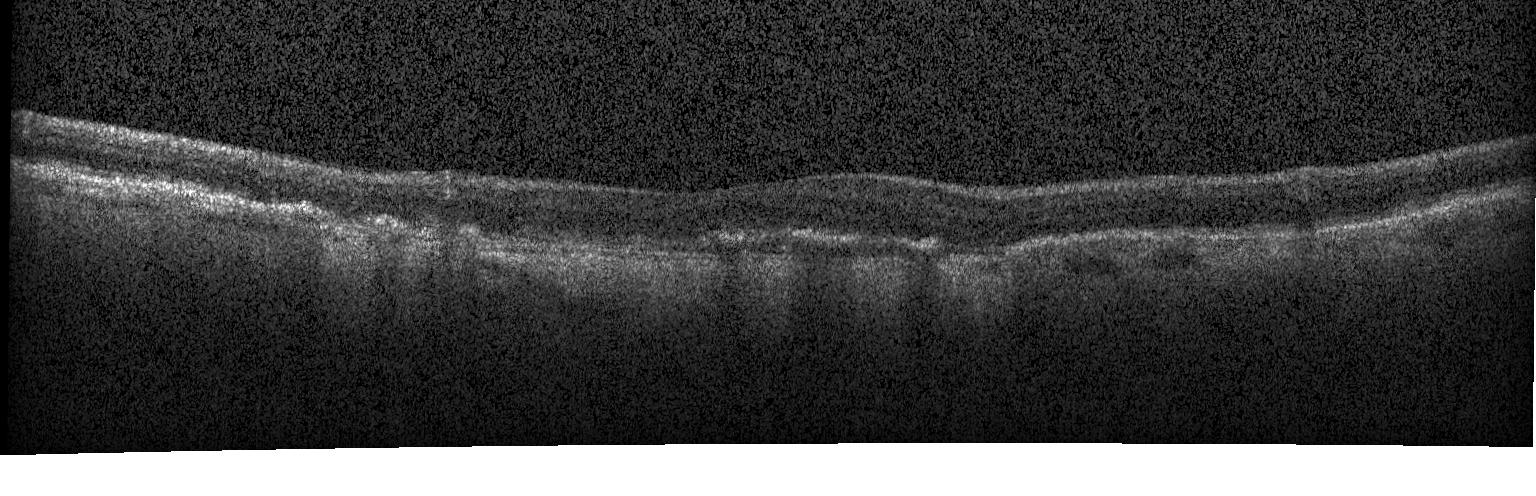

Retinal OCT cross-section showing choroidal neovascularization (CNV).